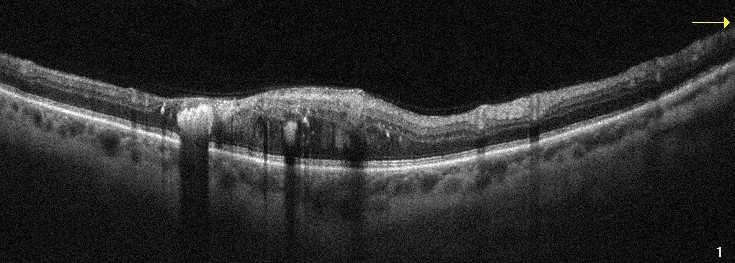 Diagnosis: diabetic macular edema (DME).